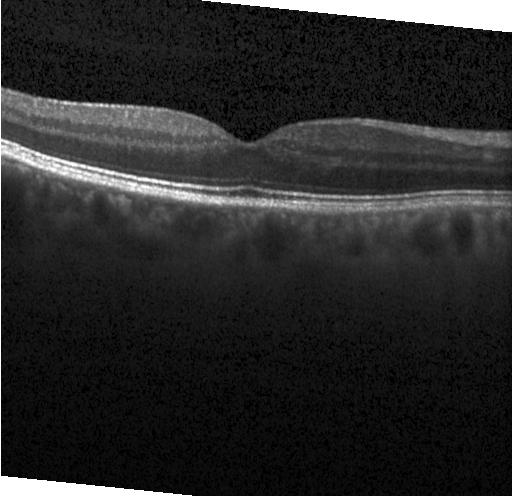 Through the macula. Optical coherence tomography B-scan. Spectral-domain optical coherence tomography. Macular OCT: no CNV, no DME, and no drusen.